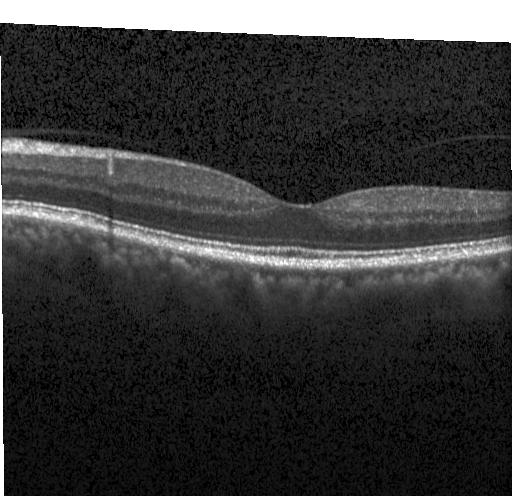
OCT B-scan showing no evidence of CNV, DME, or drusen.